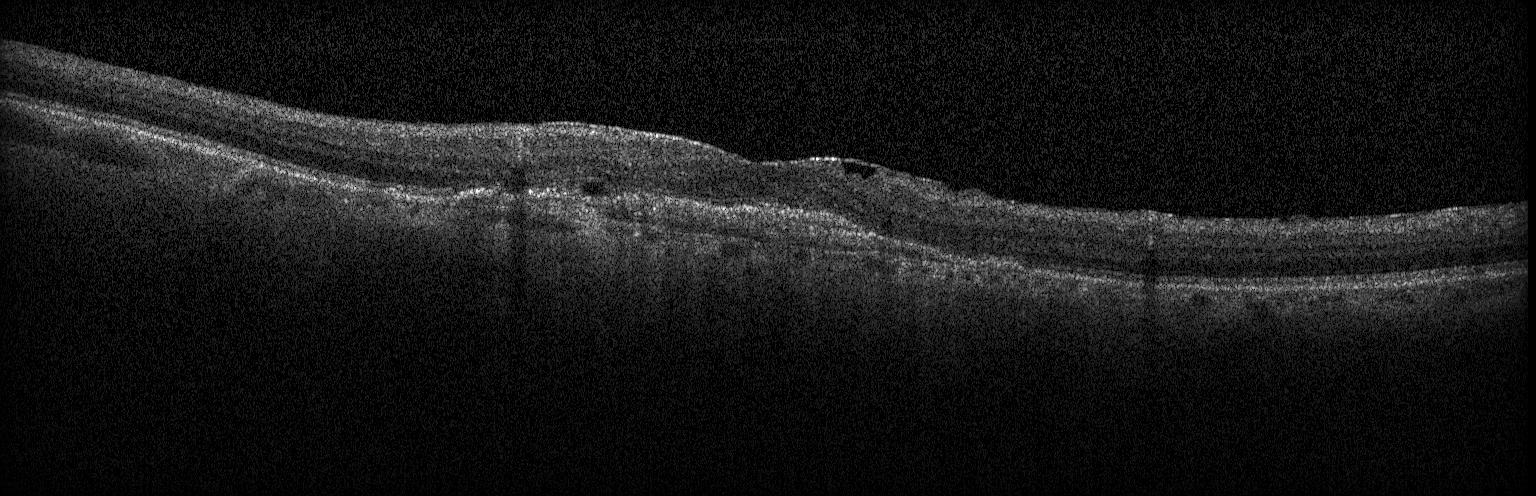

OCT finding: CNV.